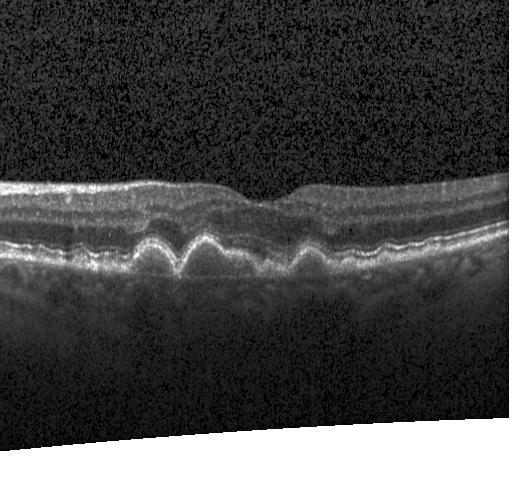 OCT B-scan showing a choroidal neovascular membrane.